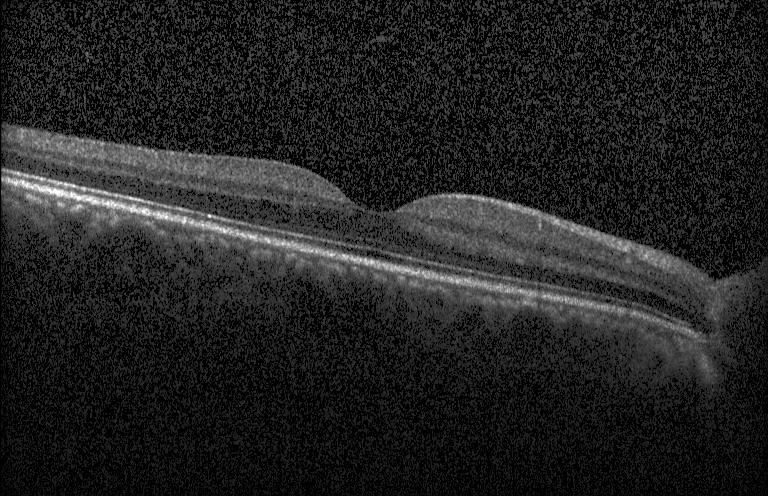 Retinal OCT cross-section
This B-scan demonstrates no evidence of choroidal neovascularization, diabetic macular edema, or drusen.